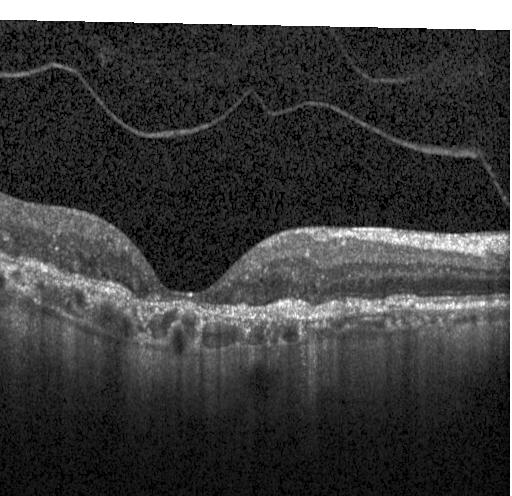 Impression: choroidal neovascularization.